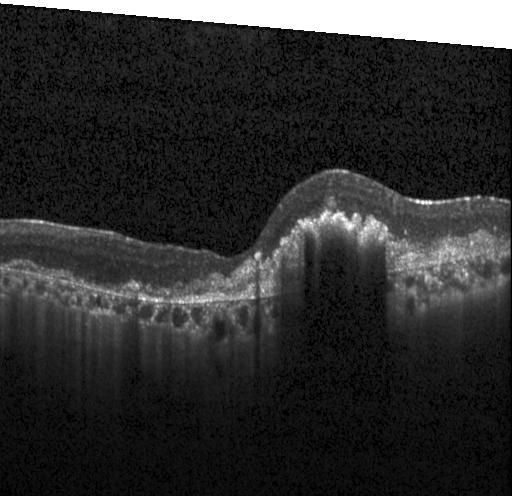 OCT B-scan showing choroidal neovascularization.